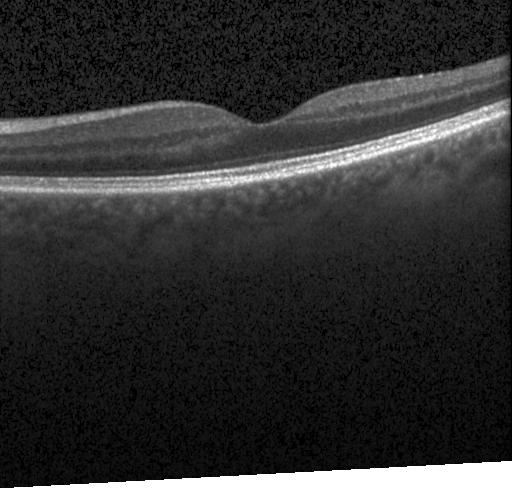 Optical coherence tomography scan. Diagnosis: no evidence of choroidal neovascularization, diabetic macular edema, or drusen.